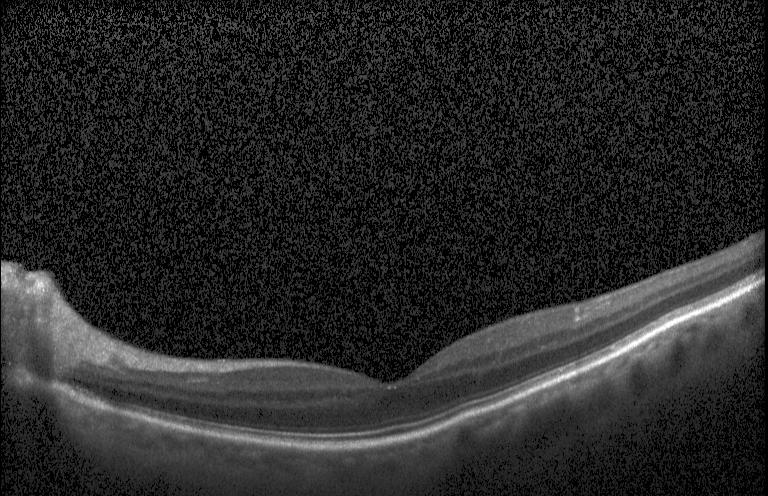
Macular OCT: no evidence of choroidal neovascularization, diabetic macular edema, or drusen.